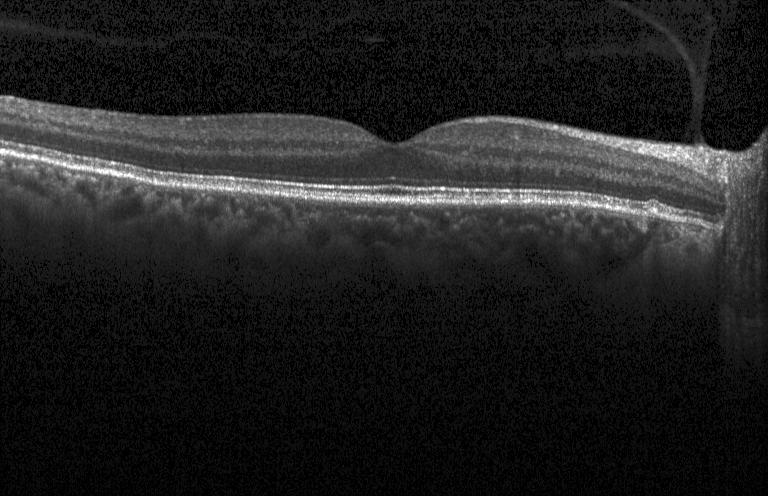

Instrument: Heidelberg Spectralis. Retinal OCT B-scan
This B-scan demonstrates sub-RPE drusenoid deposits.